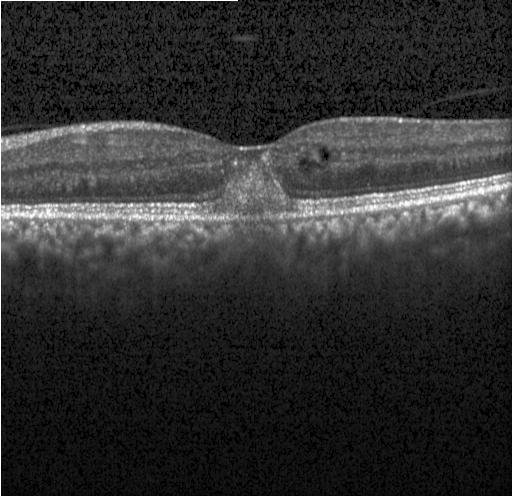 Spectral-domain OCT B-scan: choroidal neovascularization (CNV).